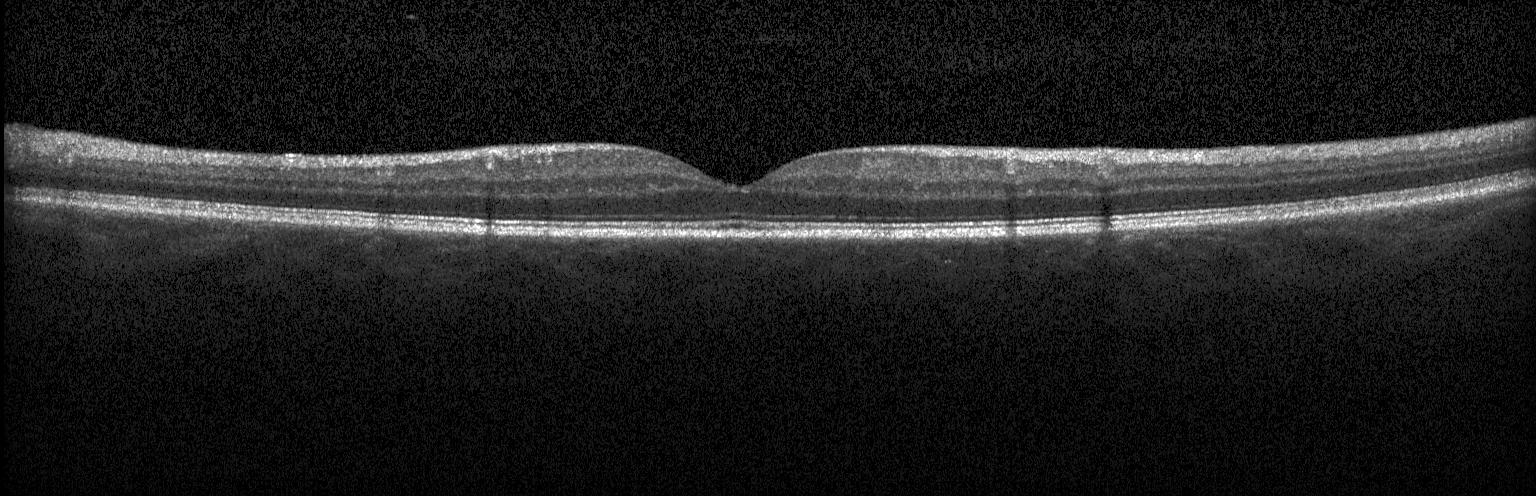 Impression: neither choroidal neovascularization, diabetic macular edema, nor drusen.